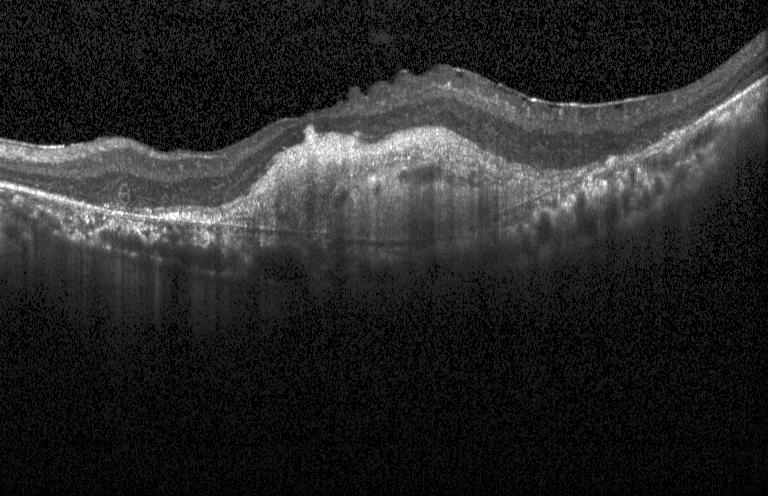 The scan shows a choroidal neovascular membrane.